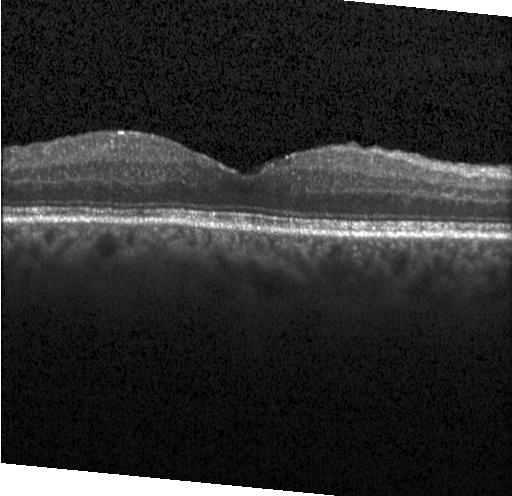 Diagnosis: neither choroidal neovascularization, diabetic macular edema, nor drusen.